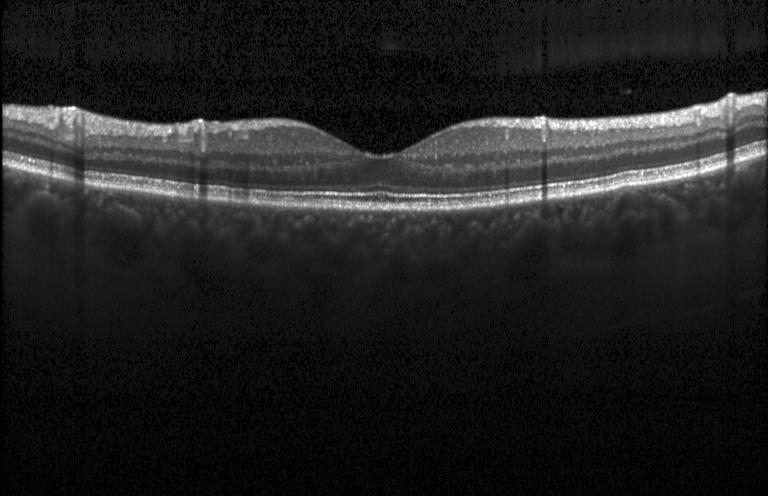 Macular OCT: no CNV, DME, or drusen.